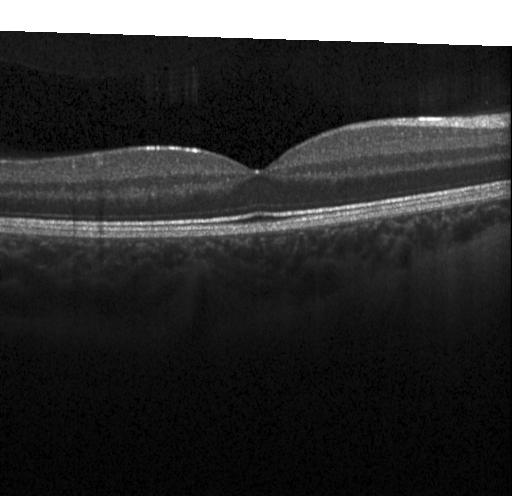 OCT line scan
Macular OCT: neither choroidal neovascularization, diabetic macular edema, nor drusen.